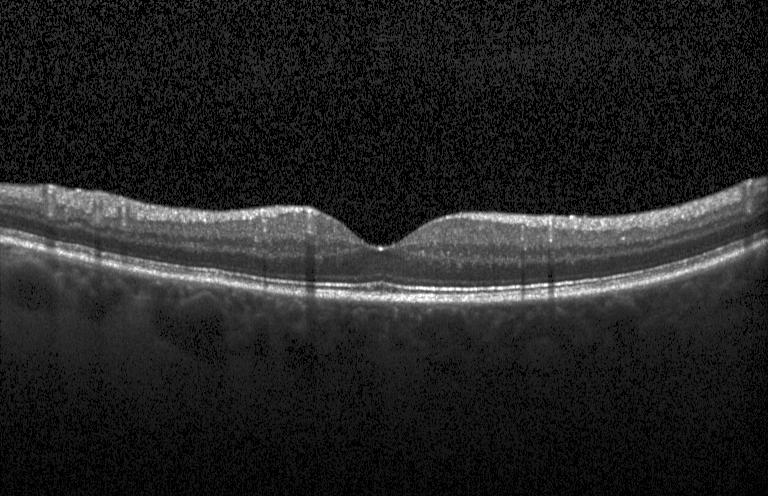 OCT B-scan showing no CNV, no DME, and no drusen.